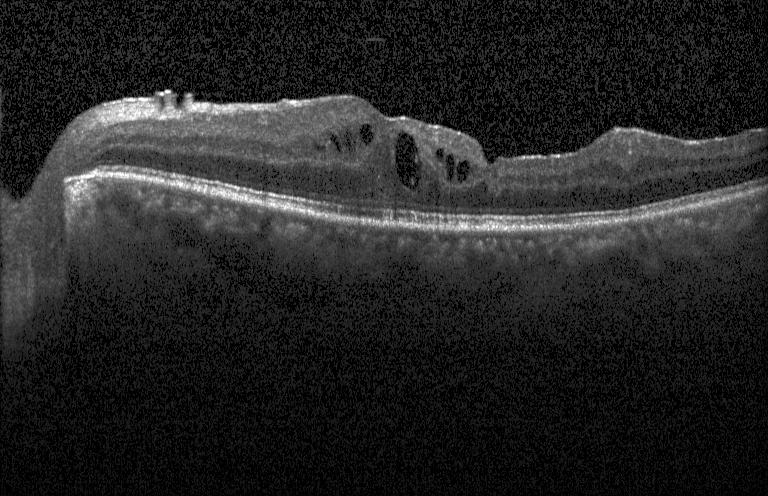

Diagnosis: diabetic macular edema.